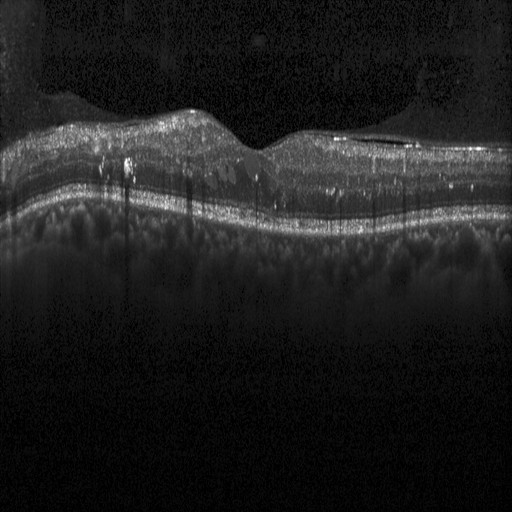 OCT line scan, acquired on a Heidelberg Spectralis.
Impression: diabetic macular edema.